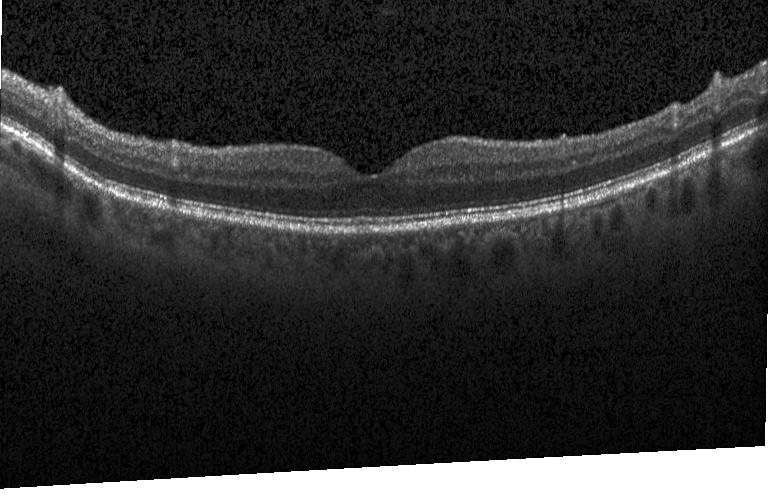

OCT scan showing neither choroidal neovascularization, diabetic macular edema, nor drusen.